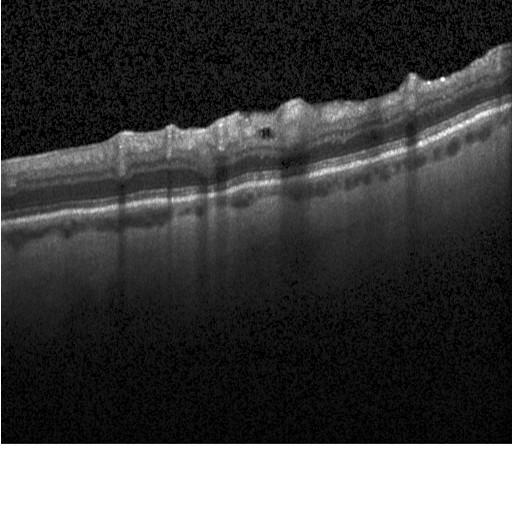

Impression: diabetic macular edema (DME).